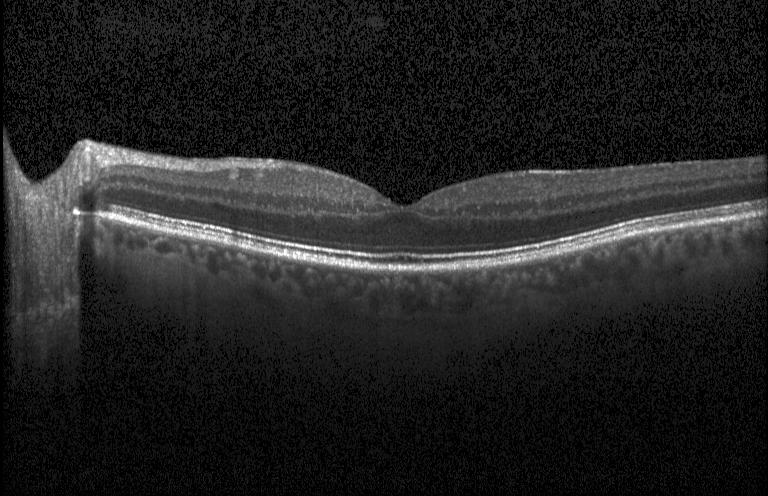 Through the macula · OCT B-scan · Heidelberg Spectralis · spectral-domain optical coherence tomography
The scan shows no CNV, DME, or drusen.